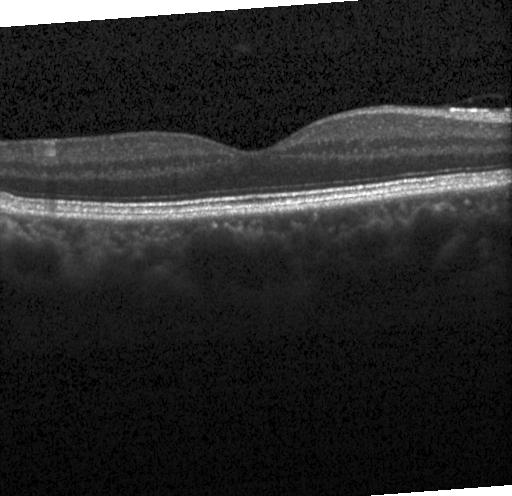 This B-scan demonstrates neither choroidal neovascularization, diabetic macular edema, nor drusen.